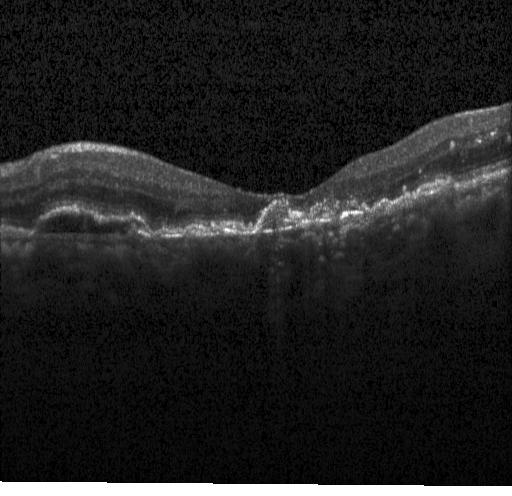
Finding: CNV.